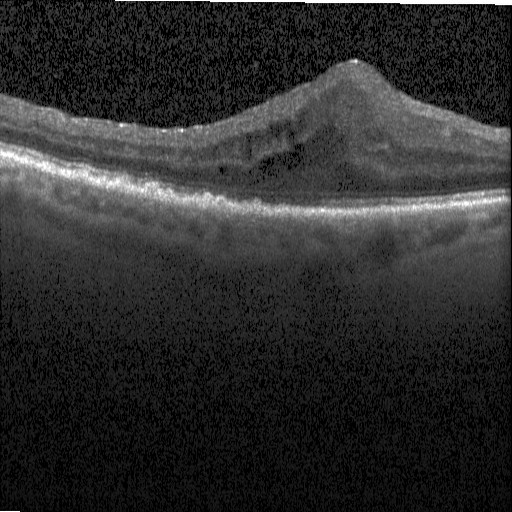 Spectral-domain OCT B-scan: DME.